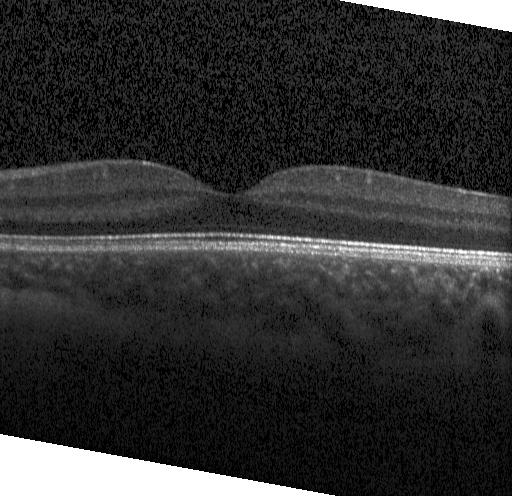

Impression: no choroidal neovascularization, diabetic macular edema, or drusen.